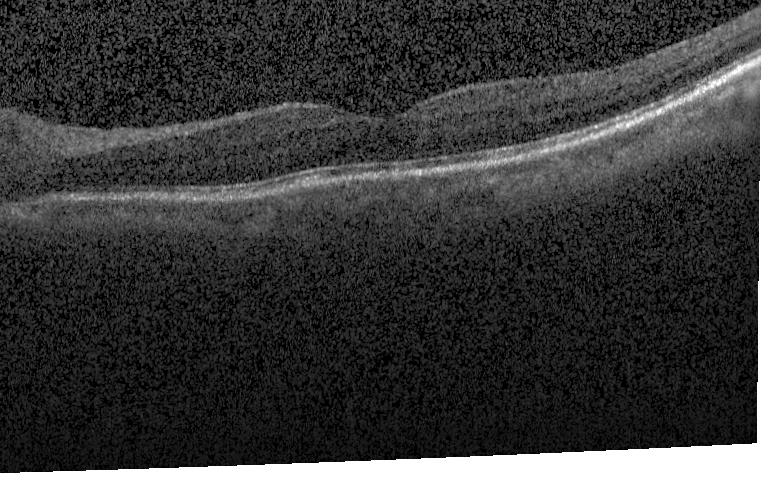 Retinal OCT cross-section showing no CNV, DME, or drusen.